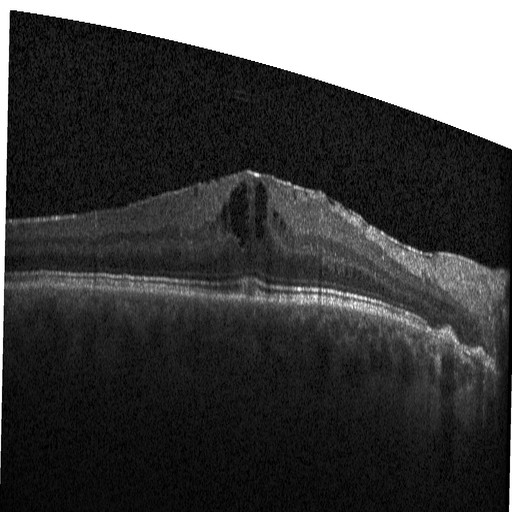

Acquired on a Heidelberg Spectralis. SD-OCT. Through the macula. Retinal OCT B-scan — DME.